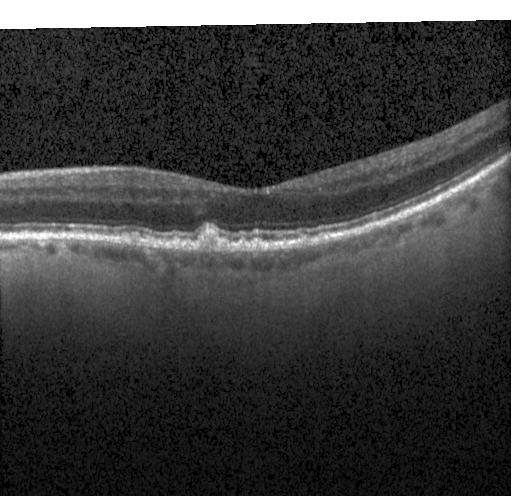
Retinal OCT cross-section — This B-scan demonstrates drusen.